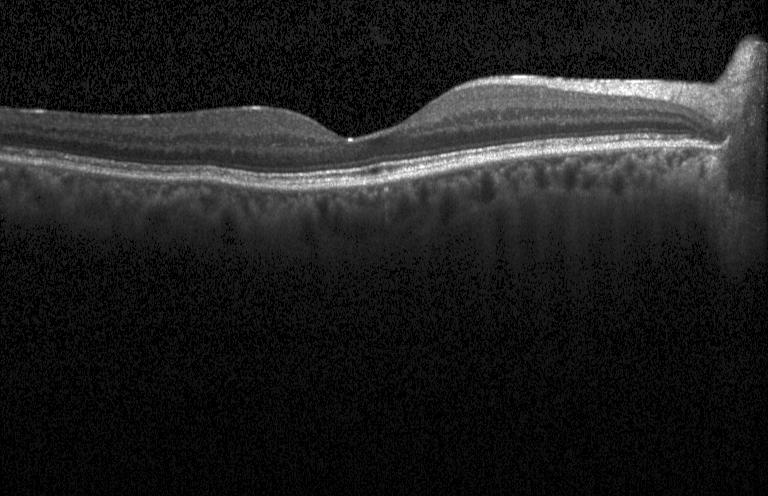

Assessment: no choroidal neovascularization, diabetic macular edema, or drusen.